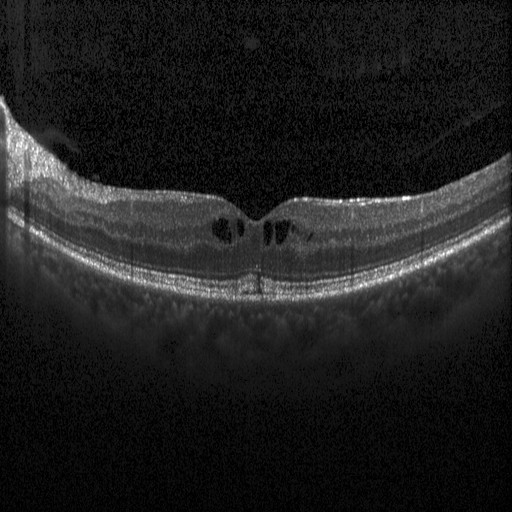 Centered on the fovea; optical coherence tomography B-scan; Heidelberg Spectralis; spectral-domain OCT
Diagnosis: diabetic macular edema (DME).